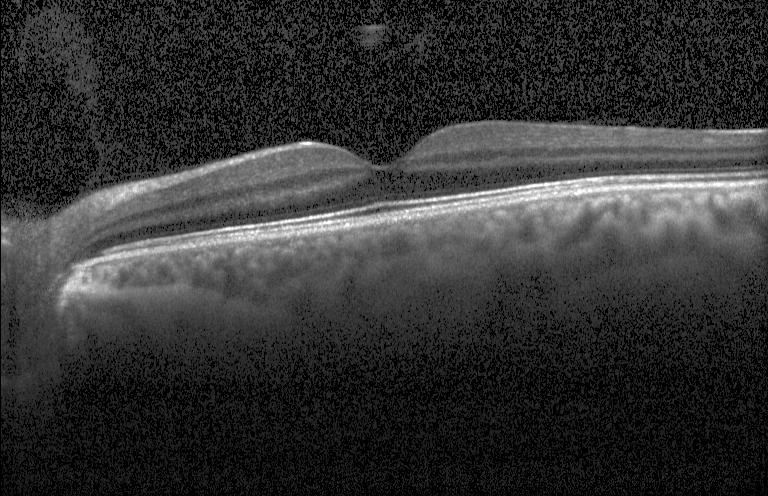 Assessment: no evidence of choroidal neovascularization, diabetic macular edema, or drusen.